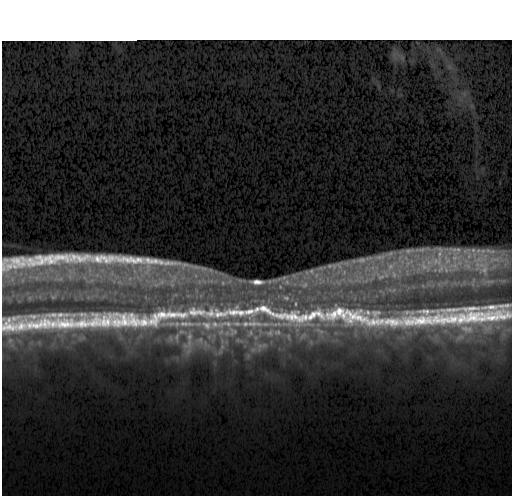 Finding: a choroidal neovascular membrane.